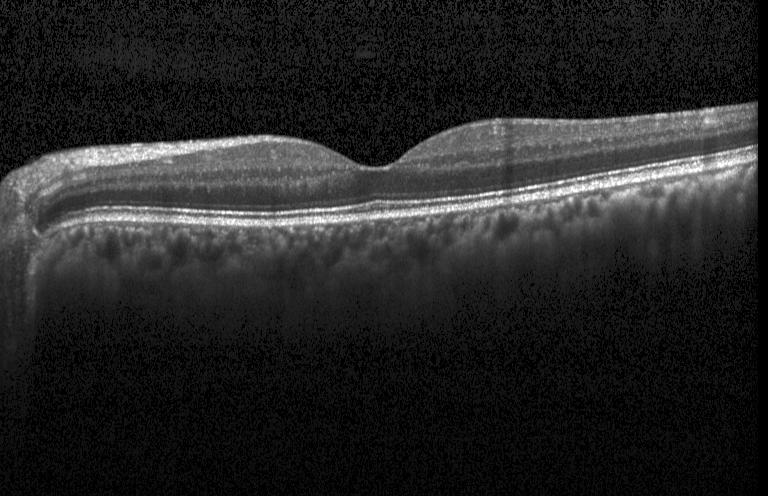

Spectral-domain optical coherence tomography; optical coherence tomography scan; Heidelberg Spectralis — No evidence of choroidal neovascularization, diabetic macular edema, or drusen.